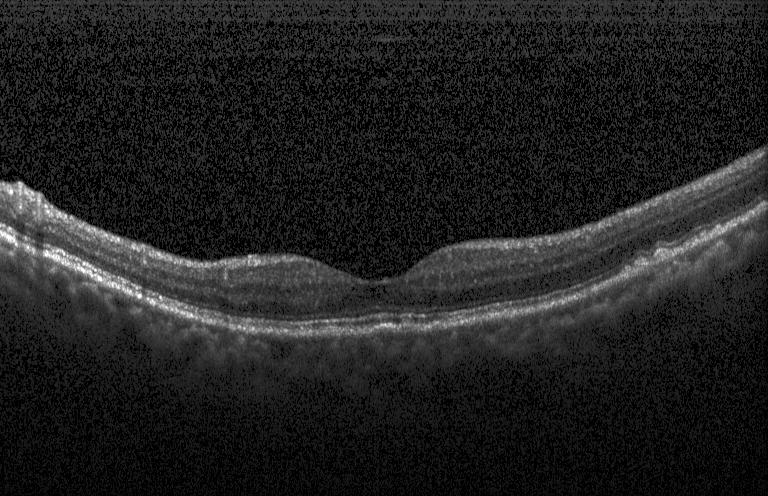 Horizontal scan through the fovea, OCT line scan. Finding: multiple drusen.